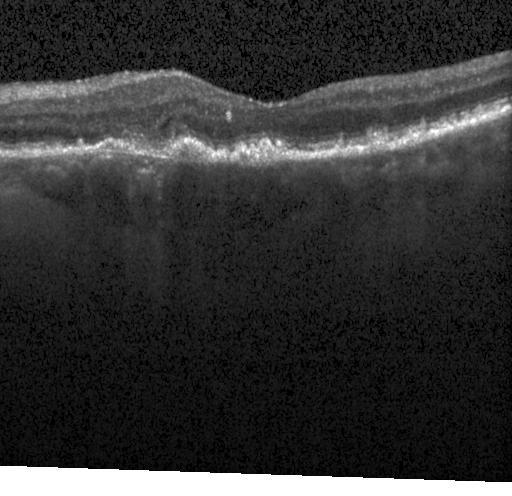 Optical coherence tomography B-scan. Instrument: Heidelberg Spectralis
OCT finding: multiple drusen.